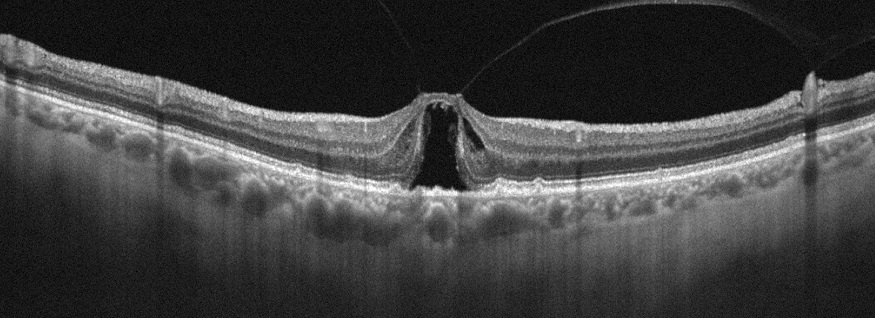

Optical coherence tomography B-scan — Finding: VID.